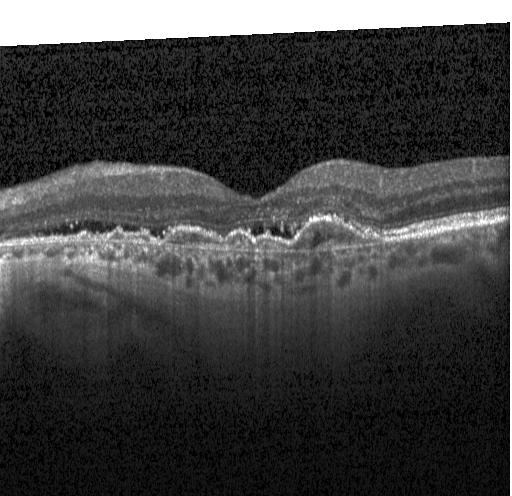 Retinal OCT B-scan. CNV.